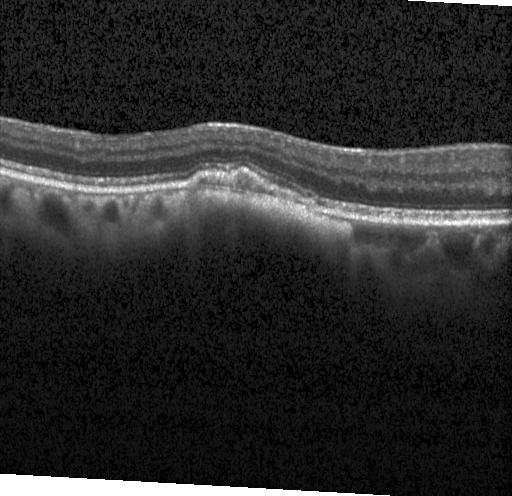

Optical coherence tomography B-scan — A choroidal neovascular membrane.